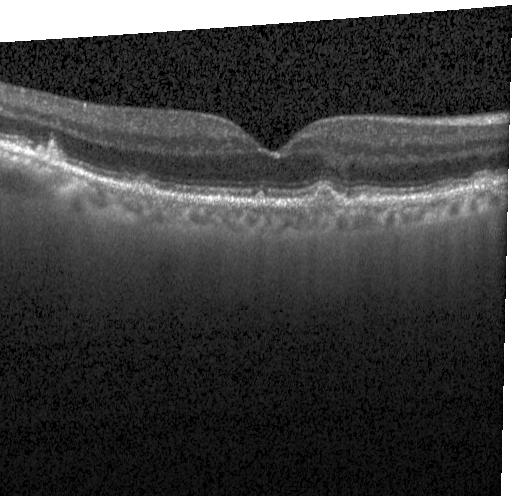
Retinal OCT B-scan, acquired on a Heidelberg Spectralis, spectral-domain OCT — Finding: multiple drusen.